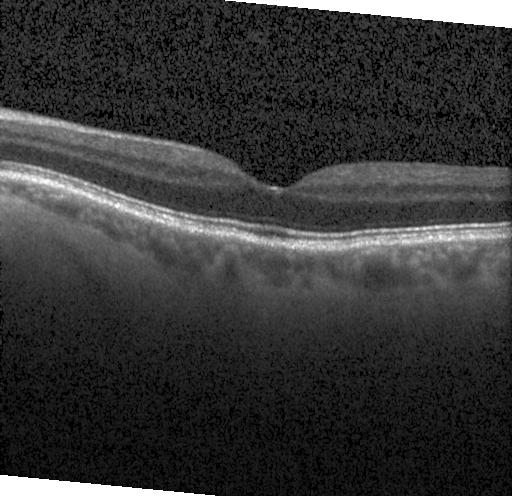 The scan shows no choroidal neovascularization, no diabetic macular edema, and no drusen.